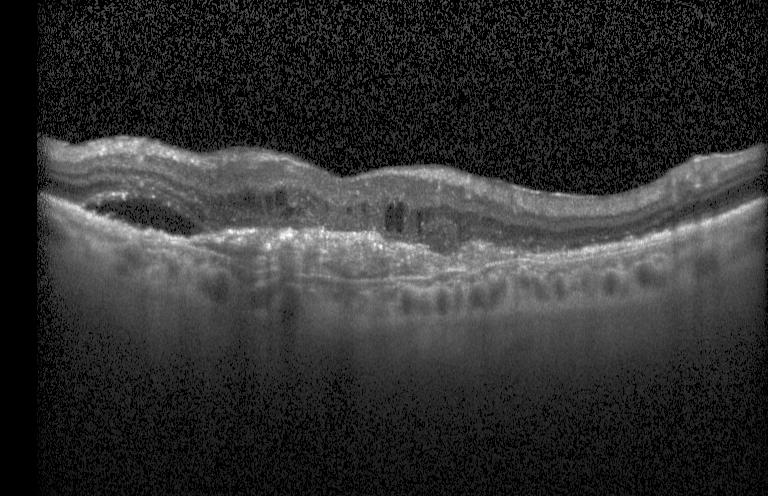 Diagnosis: a choroidal neovascular membrane.